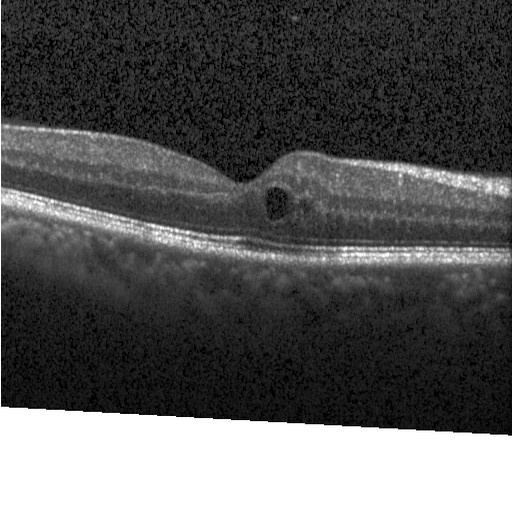

Through the macula. OCT B-scan. Spectral-domain optical coherence tomography — Impression: diabetic macular edema.